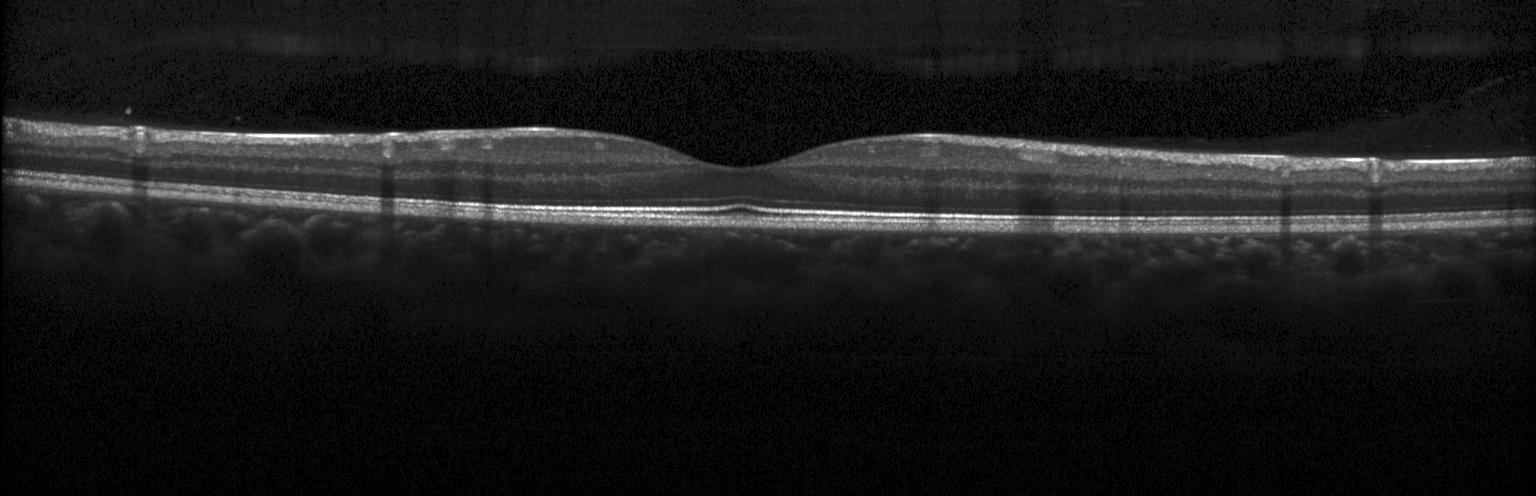
OCT line scan. Assessment: no choroidal neovascularization, no diabetic macular edema, and no drusen.